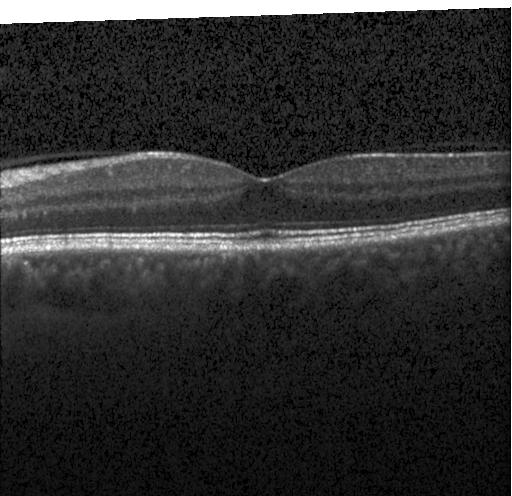 Finding: no CNV, no DME, and no drusen.